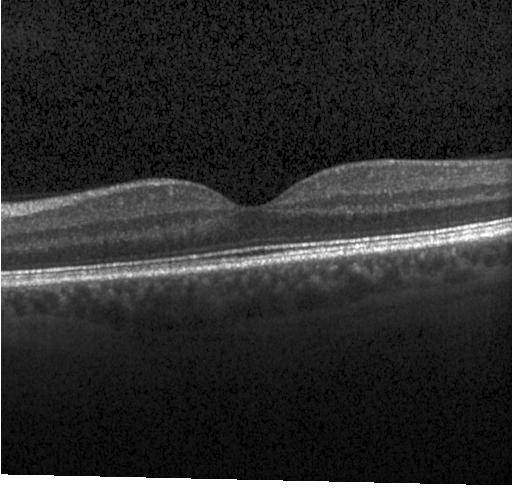 Diagnosis: no evidence of choroidal neovascularization, diabetic macular edema, or drusen.